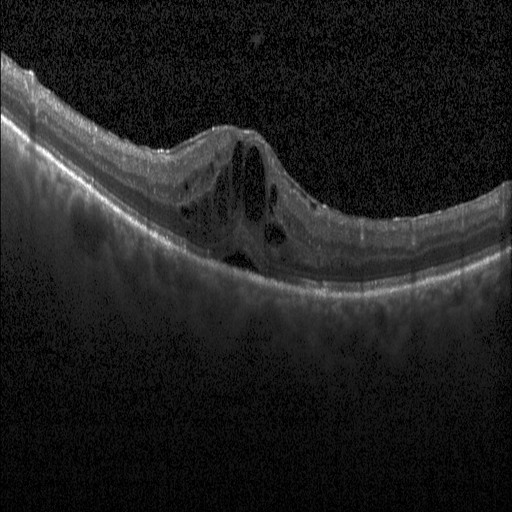

SD-OCT · optical coherence tomography B-scan — Finding: diabetic macular edema (DME).